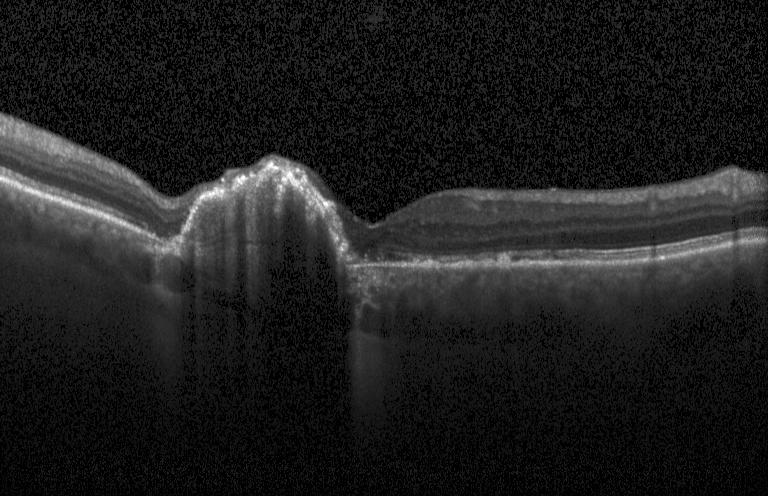

Optical coherence tomography scan · acquired on a Heidelberg Spectralis
Dx: choroidal neovascularization.